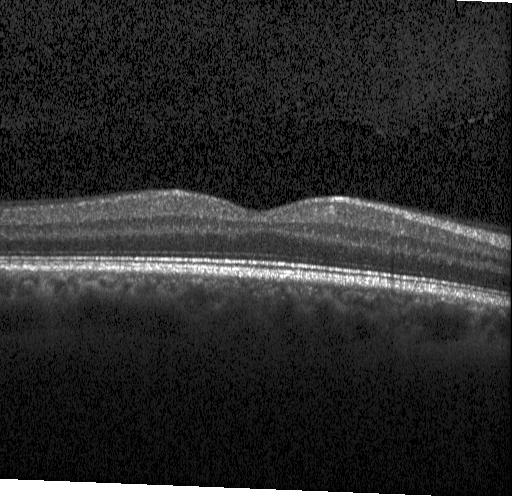 Retinal OCT cross-section showing no choroidal neovascularization, no diabetic macular edema, and no drusen.